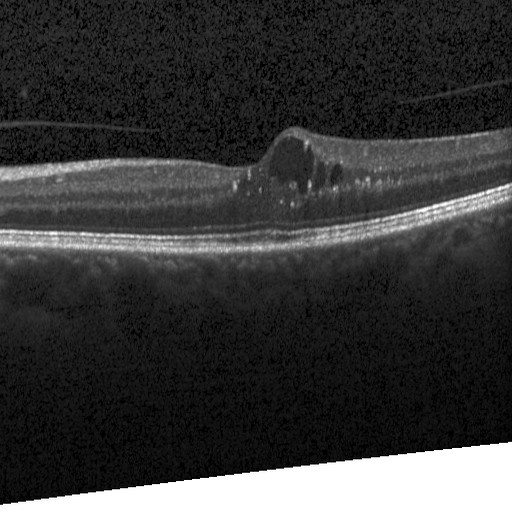

OCT finding: diabetic macular edema.